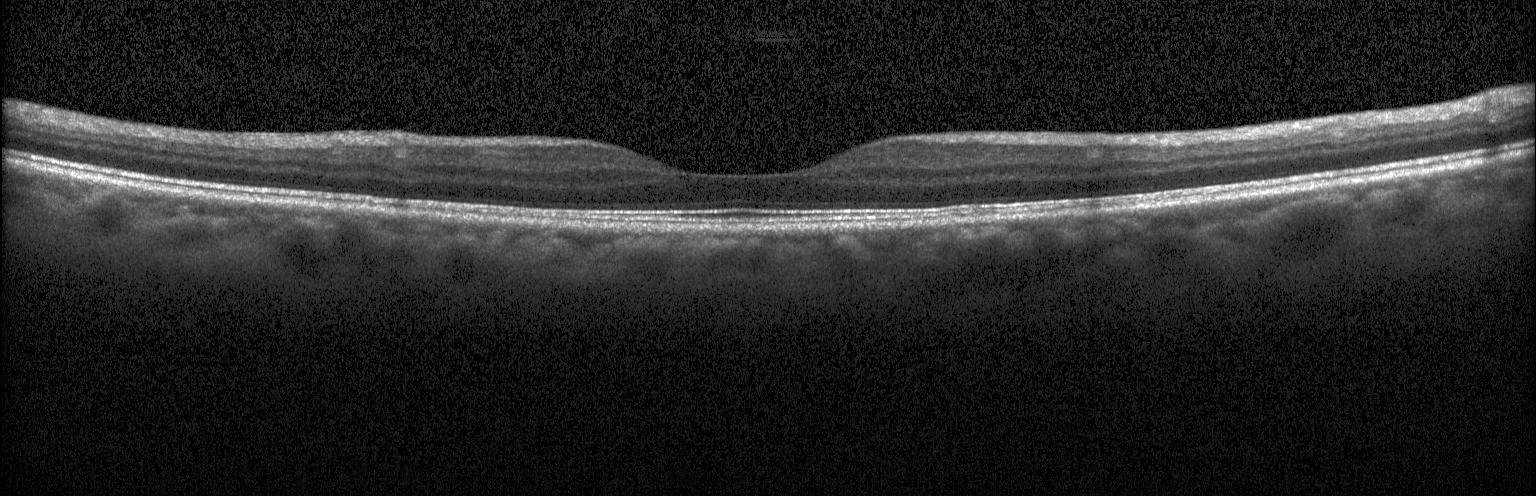 Dx: no CNV, DME, or drusen.